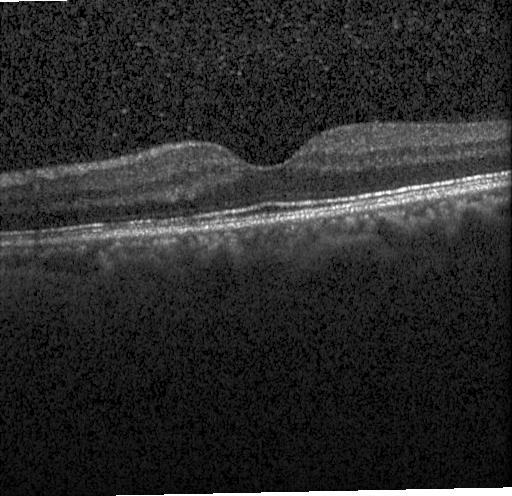 Retinal OCT cross-section; acquired on a Heidelberg Spectralis; horizontal scan through the fovea
Impression: no evidence of choroidal neovascularization, diabetic macular edema, or drusen.